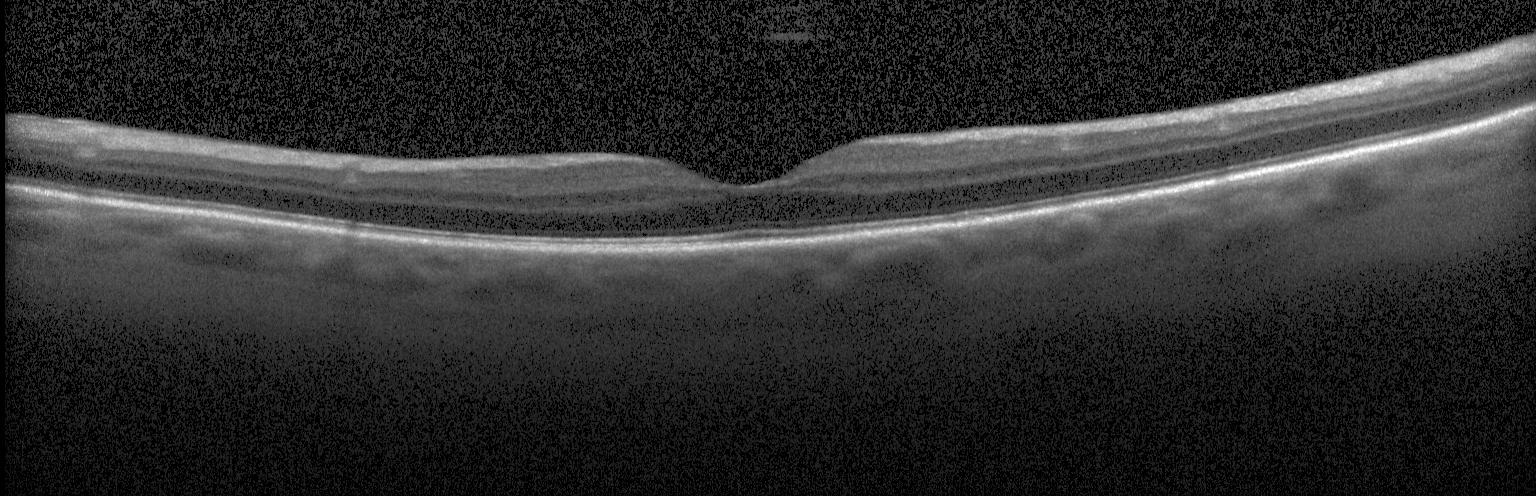

Retinal OCT cross-section.
No CNV, no DME, and no drusen.